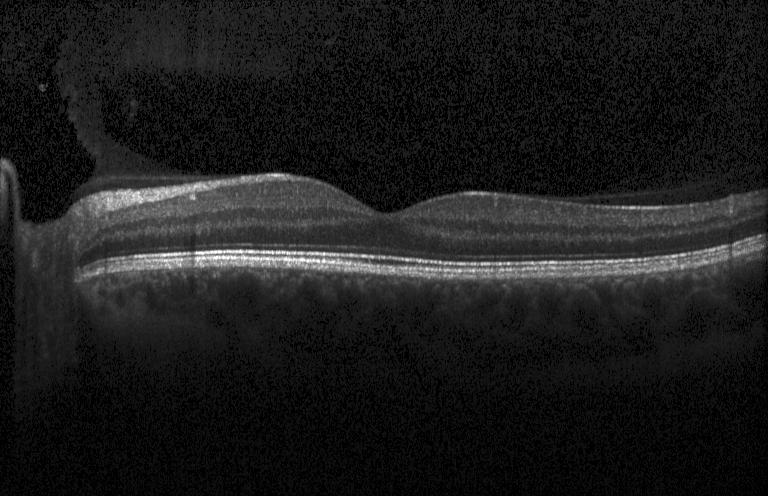 Spectral-domain optical coherence tomography · optical coherence tomography scan · macular scan.
OCT finding: no choroidal neovascularization, no diabetic macular edema, and no drusen.